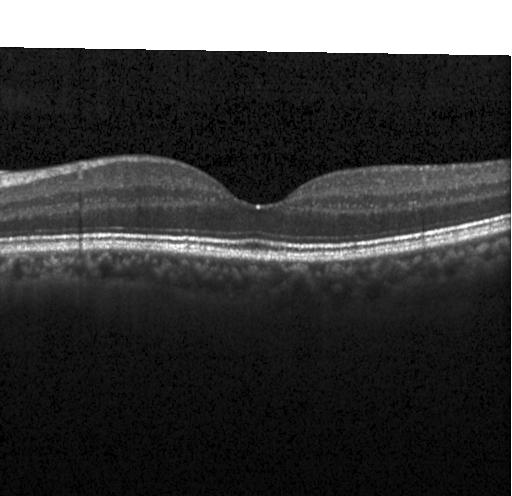
Macular OCT demonstrating no choroidal neovascularization, no diabetic macular edema, and no drusen.